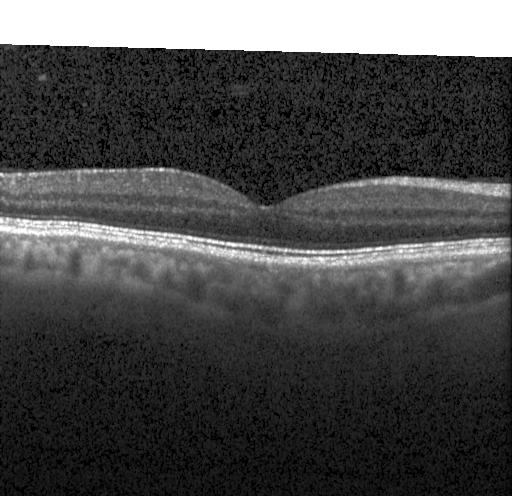
Impression: neither choroidal neovascularization, diabetic macular edema, nor drusen.